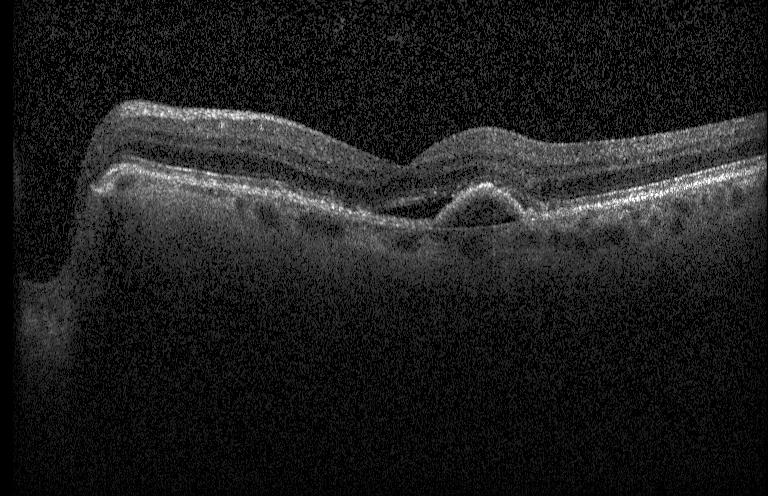
Finding: a choroidal neovascular membrane.